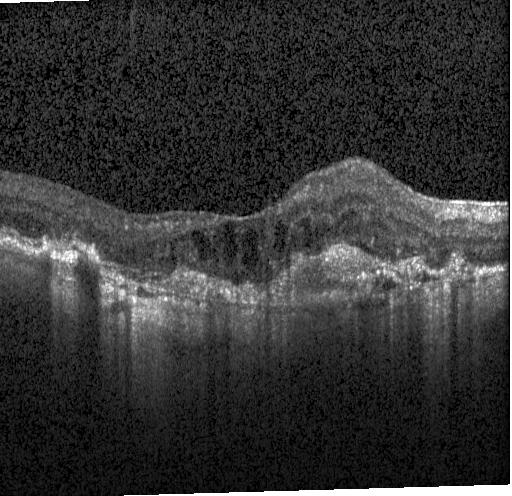

Optical coherence tomography scan. Finding: a choroidal neovascular membrane.